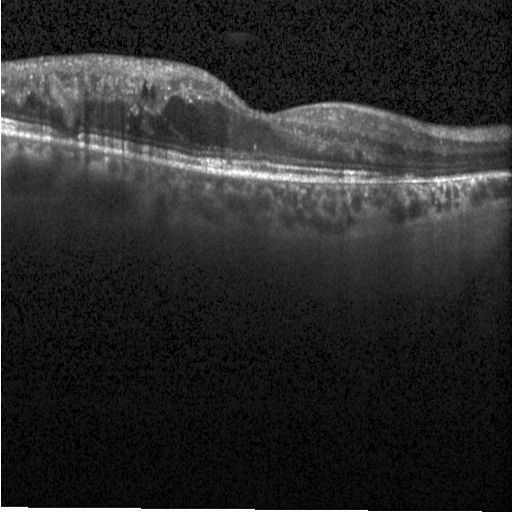

Spectral-domain OCT · Heidelberg Spectralis · OCT line scan · horizontal scan through the fovea. Impression: diabetic macular edema.